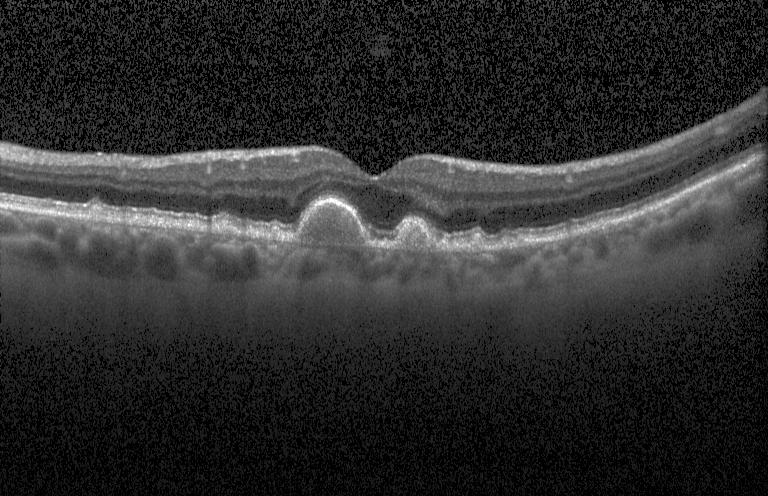

Heidelberg Spectralis; centered on the fovea; optical coherence tomography scan — Macular OCT: drusen.